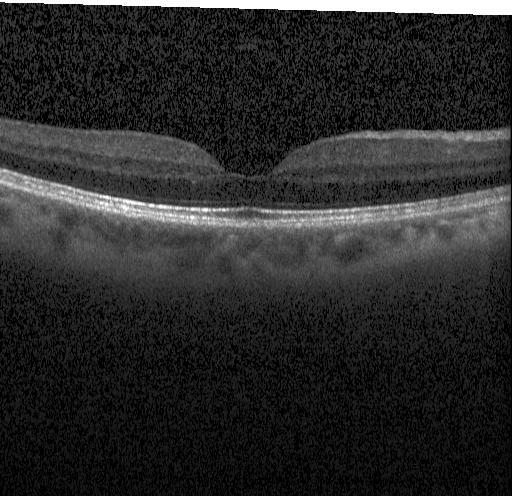
Horizontal scan through the fovea · retinal OCT cross-section · spectral-domain optical coherence tomography — The scan shows no CNV, no DME, and no drusen.